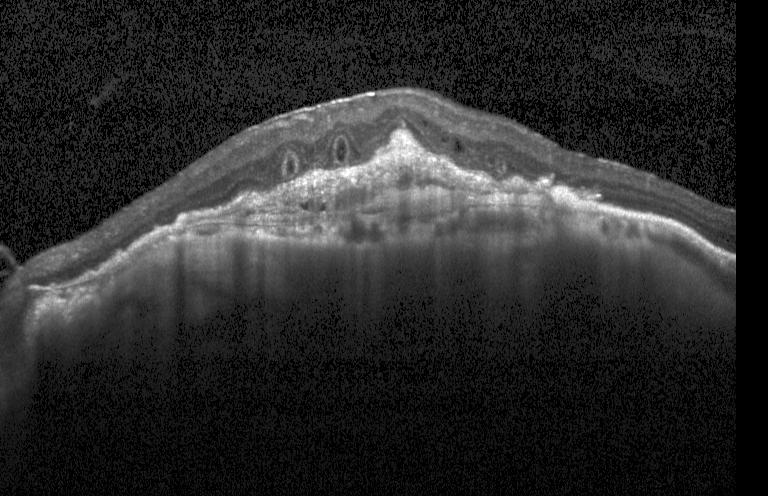
Optical coherence tomography scan — OCT finding: a choroidal neovascular membrane.